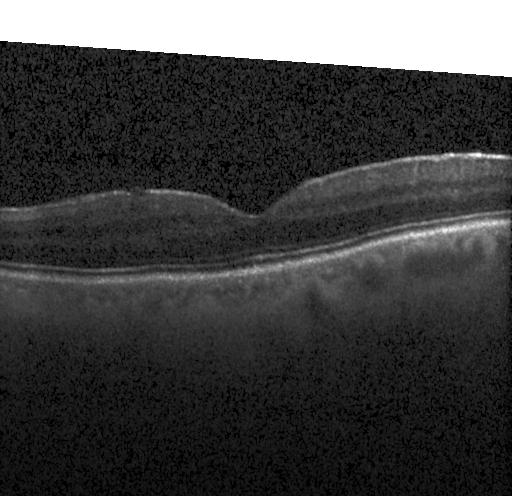

Diagnosis: no choroidal neovascularization, no diabetic macular edema, and no drusen.